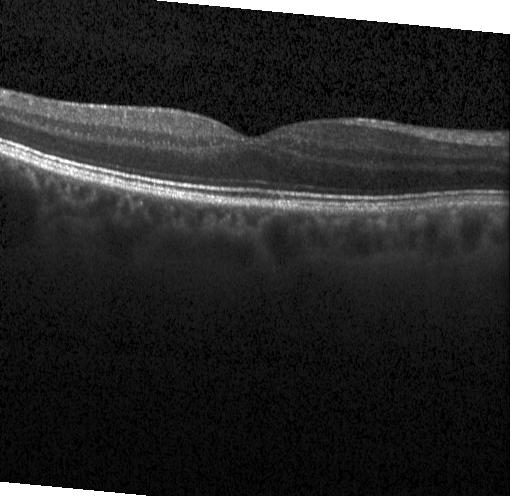 Centered on the fovea, spectral-domain optical coherence tomography, OCT line scan — This B-scan demonstrates no evidence of choroidal neovascularization, diabetic macular edema, or drusen.